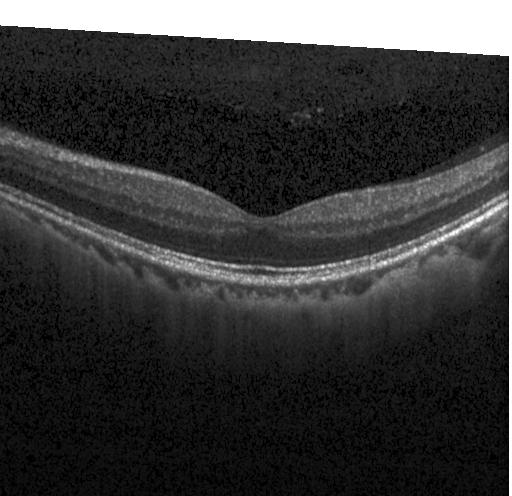 Spectral-domain OCT. Optical coherence tomography scan.
Assessment: neither choroidal neovascularization, diabetic macular edema, nor drusen.